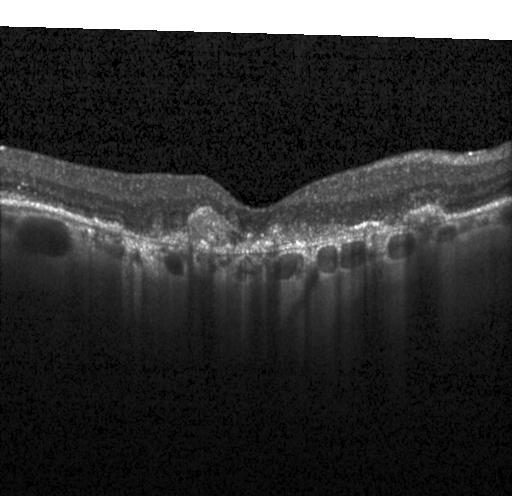 OCT scan showing choroidal neovascularization.